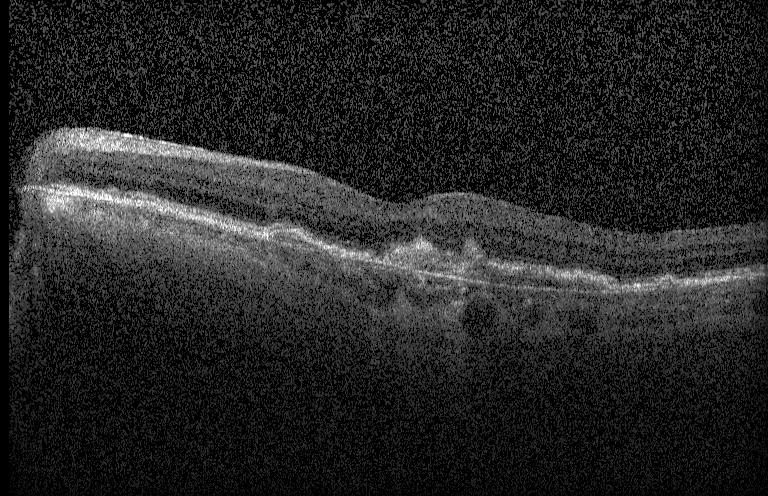
Finding: a choroidal neovascular membrane.